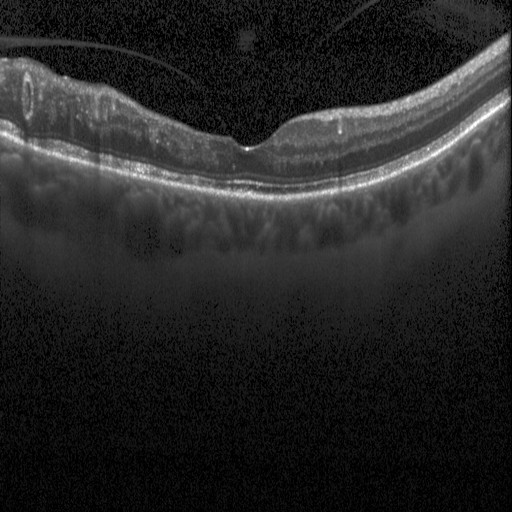 Macular OCT demonstrating DME.